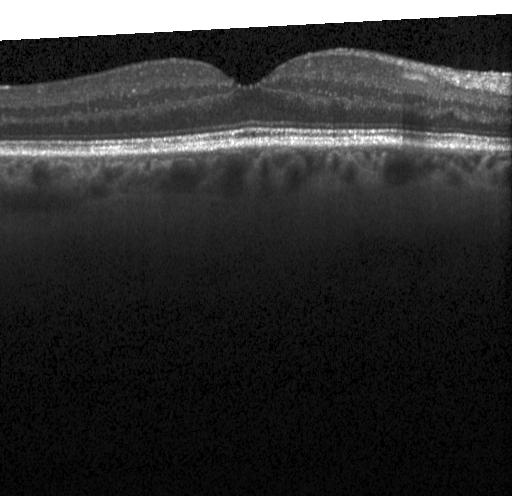

OCT B-scan — The scan shows no choroidal neovascularization, diabetic macular edema, or drusen.